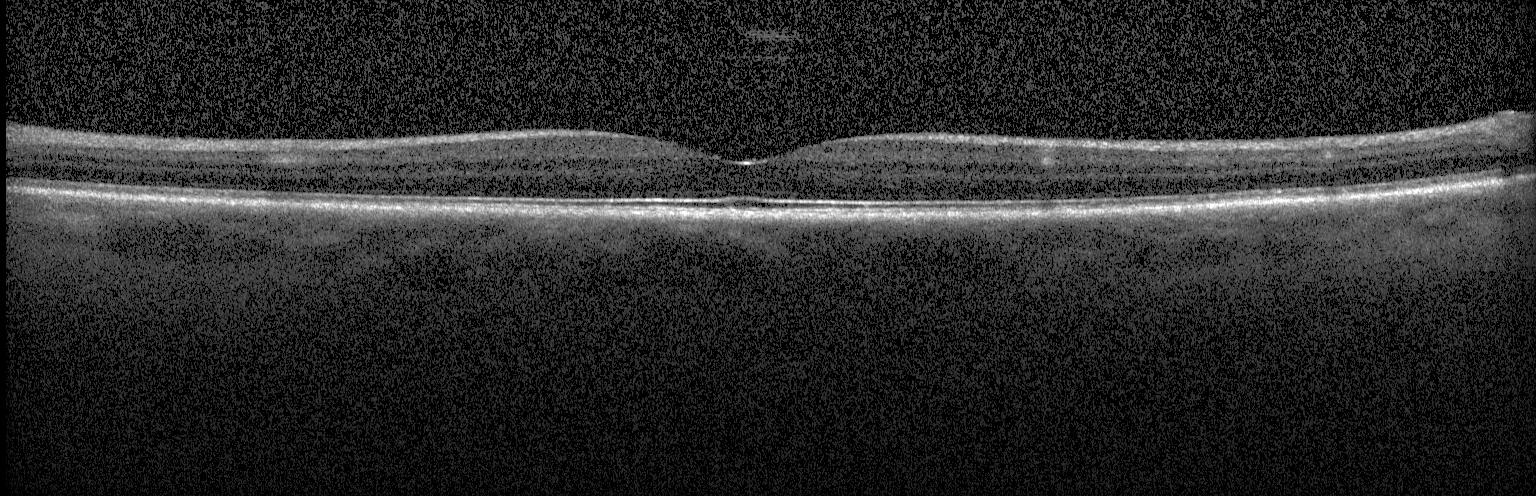

OCT finding: no choroidal neovascularization, diabetic macular edema, or drusen.